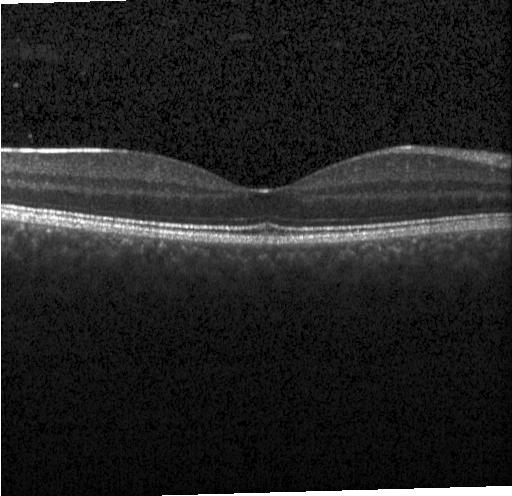

Heidelberg Spectralis OCT system. Optical coherence tomography B-scan. Centered on the fovea. SD-OCT — No evidence of CNV, DME, or drusen.